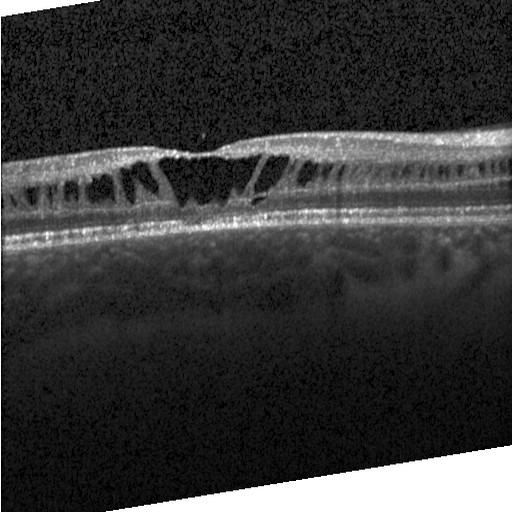 Impression: DME.